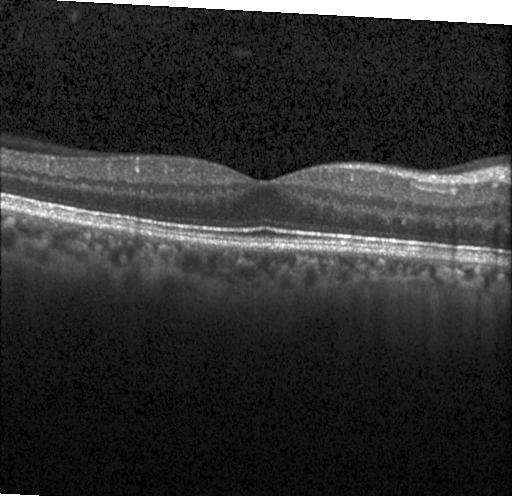 Finding: no choroidal neovascularization, diabetic macular edema, or drusen.